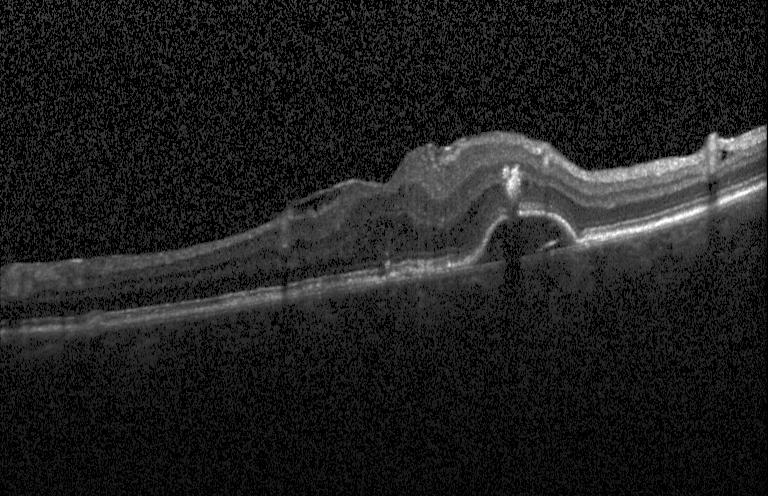

Optical coherence tomography B-scan.
Impression: choroidal neovascularization (CNV).